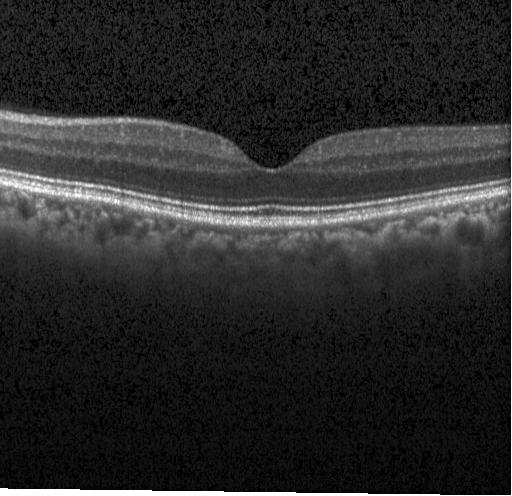 Assessment: no CNV, no DME, and no drusen.